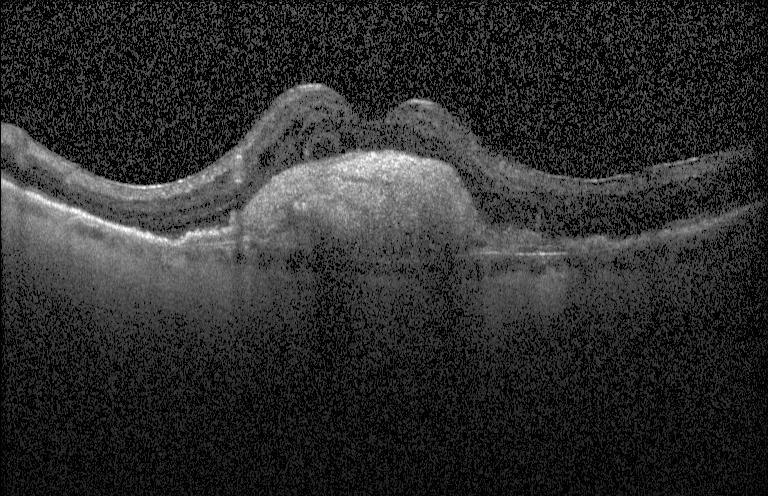 Retinal OCT B-scan — This B-scan demonstrates a choroidal neovascular membrane.